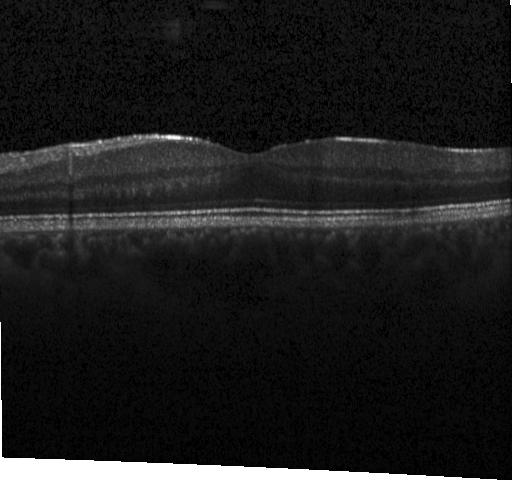

Optical coherence tomography scan · spectral-domain optical coherence tomography · Heidelberg Spectralis OCT system · fovea-centered
Diagnosis: no CNV, DME, or drusen.